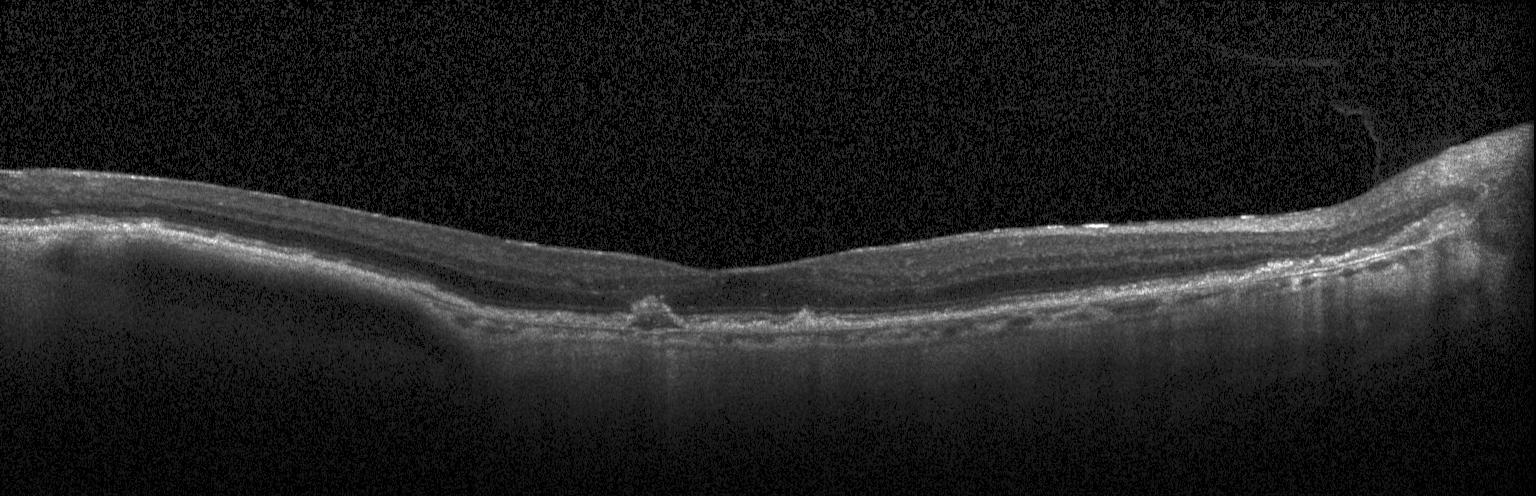
Centered on the fovea, spectral-domain OCT, retinal OCT cross-section, Heidelberg Spectralis OCT system.
This B-scan demonstrates CNV.